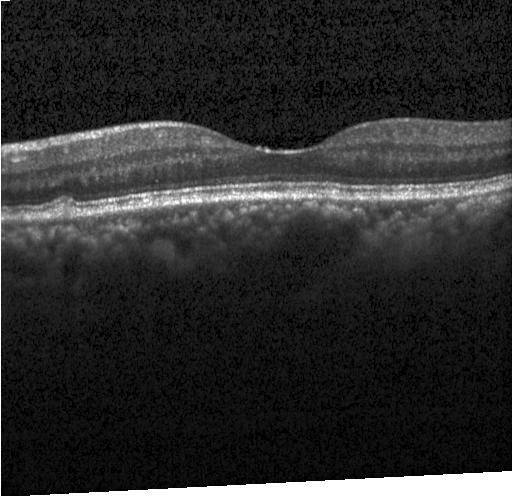
Assessment: drusen.